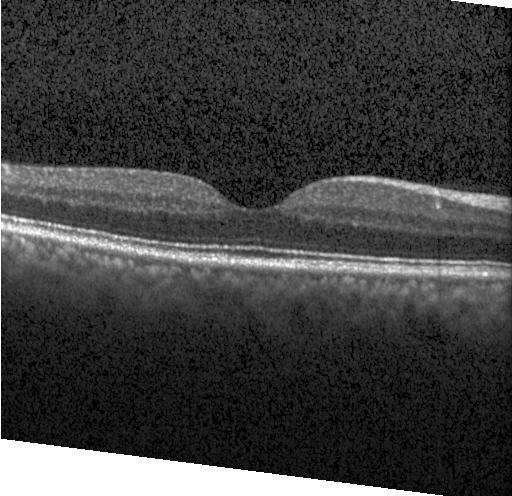

Heidelberg Spectralis OCT system. Optical coherence tomography scan. Finding: neither choroidal neovascularization, diabetic macular edema, nor drusen.